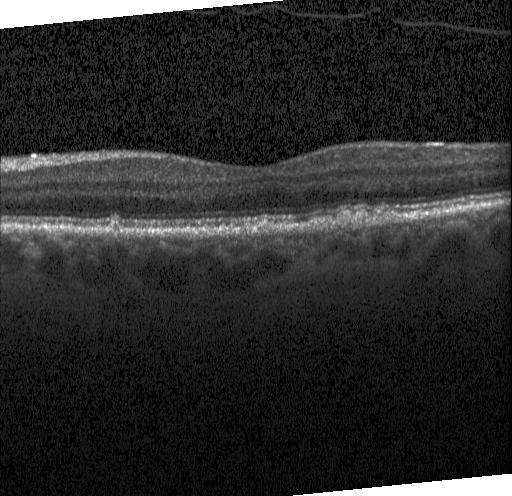
Macular OCT: drusen.